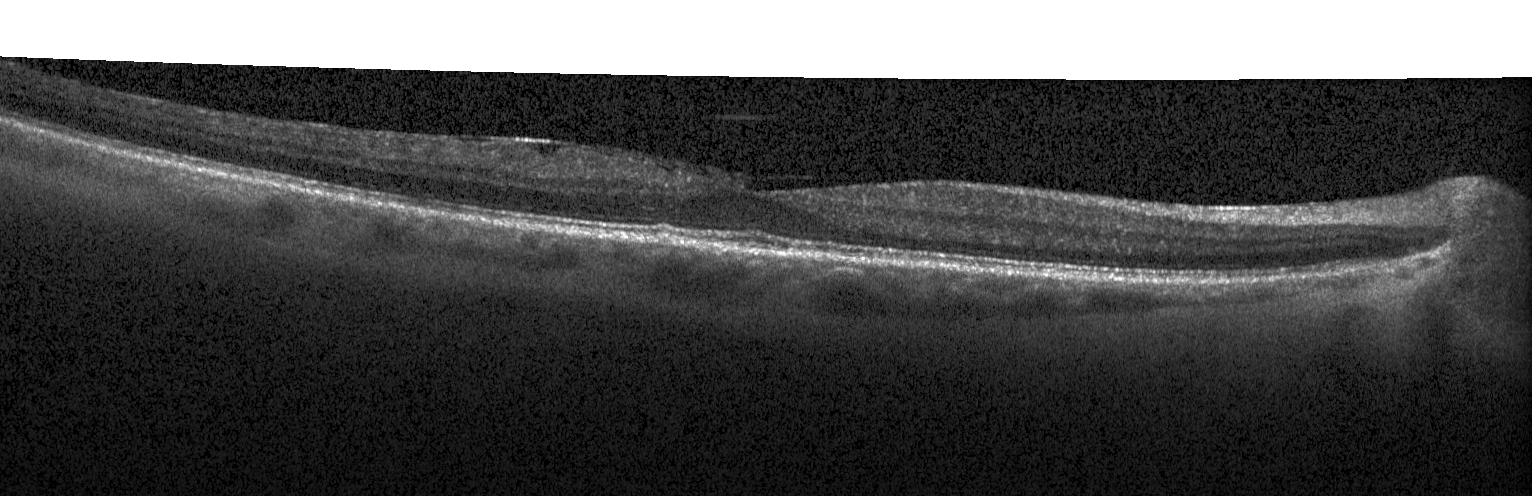

Retinal OCT B-scan, acquired on a Heidelberg Spectralis, spectral-domain optical coherence tomography — Assessment: drusen.